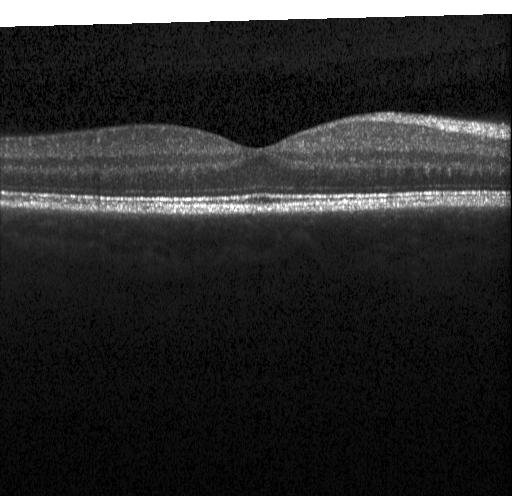
Fovea-centered. Retinal OCT B-scan. SD-OCT. Instrument: Heidelberg Spectralis. Finding: neither choroidal neovascularization, diabetic macular edema, nor drusen.